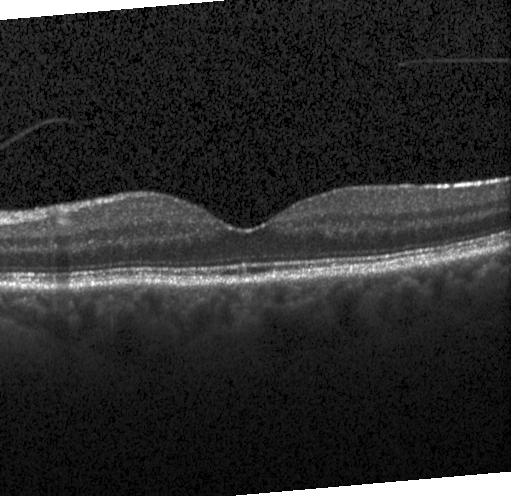

Heidelberg Spectralis OCT system, SD-OCT, OCT line scan, through the macula — Assessment: no choroidal neovascularization, diabetic macular edema, or drusen.